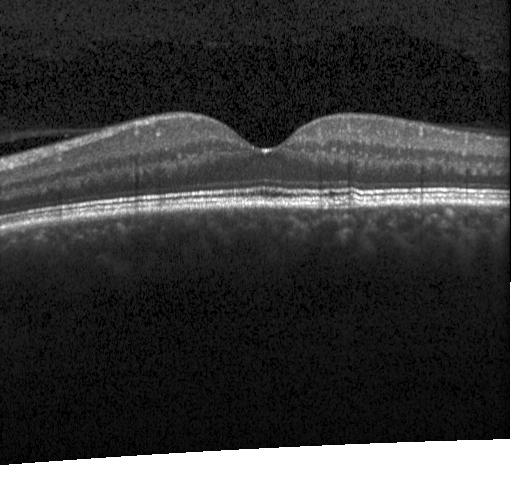
SD-OCT · optical coherence tomography scan · Heidelberg Spectralis. The scan shows multiple drusen.